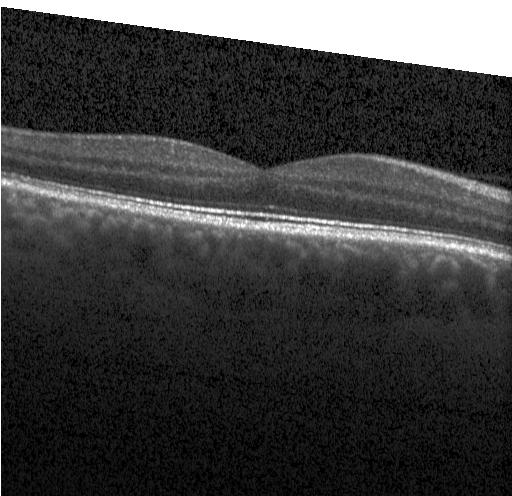
OCT B-scan showing no choroidal neovascularization, diabetic macular edema, or drusen.